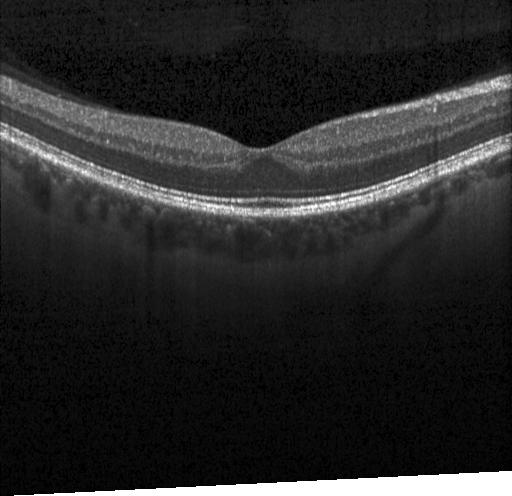

Retinal OCT cross-section showing no evidence of CNV, DME, or drusen.